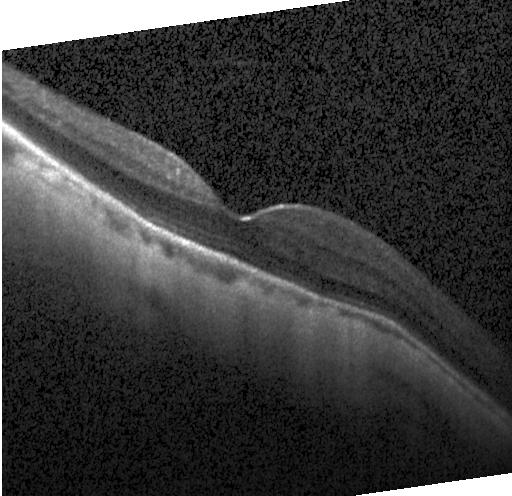

Spectral-domain OCT B-scan: neither choroidal neovascularization, diabetic macular edema, nor drusen.